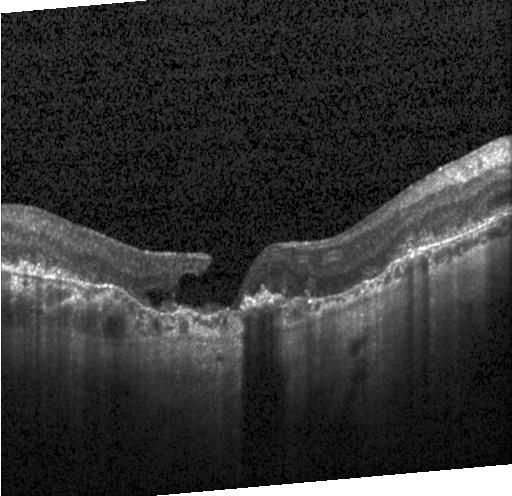

Impression: a choroidal neovascular membrane.